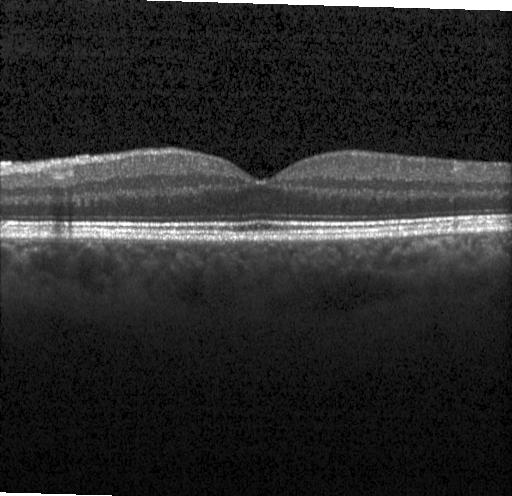

Optical coherence tomography B-scan
Dx: neither choroidal neovascularization, diabetic macular edema, nor drusen.